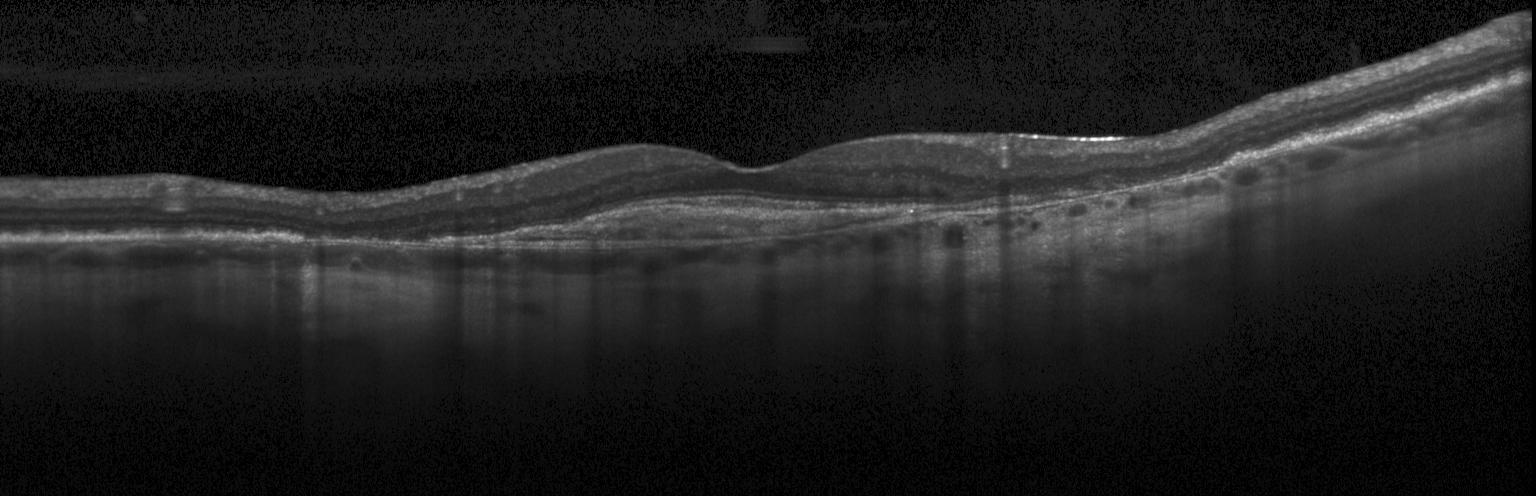 Heidelberg Spectralis. Spectral-domain OCT. Optical coherence tomography B-scan. Fovea-centered.
This B-scan demonstrates choroidal neovascularization (CNV).